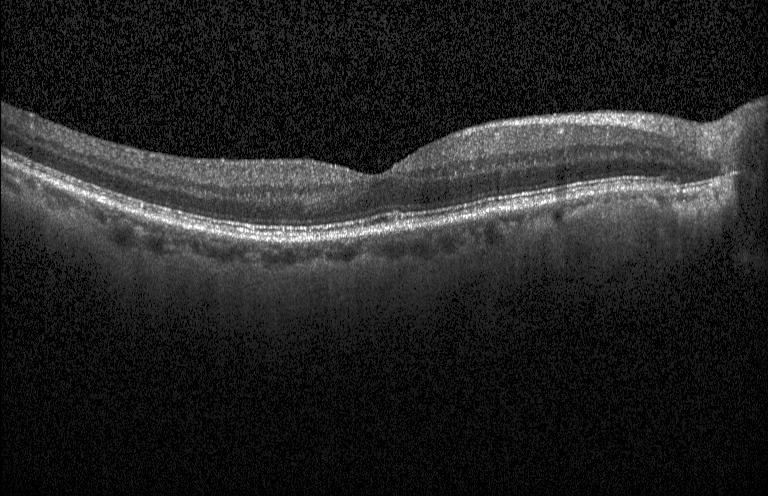
The scan shows no choroidal neovascularization, no diabetic macular edema, and no drusen.